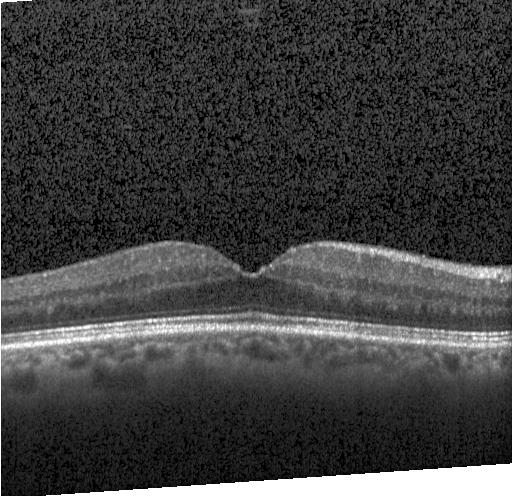 OCT finding: no CNV, no DME, and no drusen.